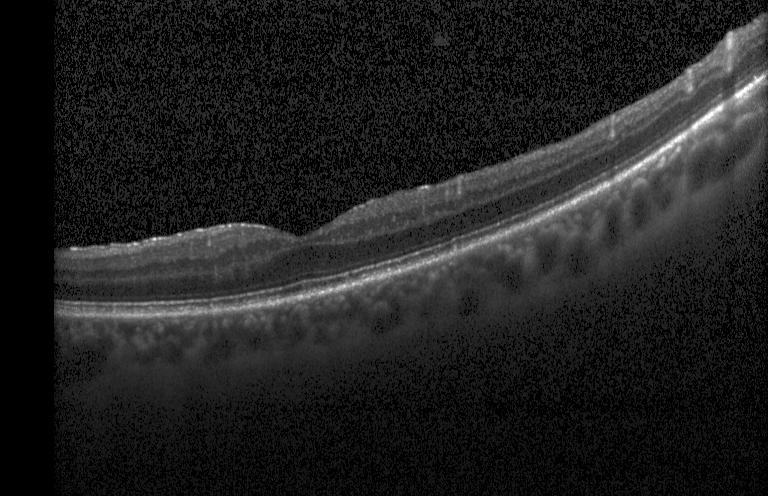 OCT line scan. Spectral-domain optical coherence tomography — Impression: no CNV, DME, or drusen.